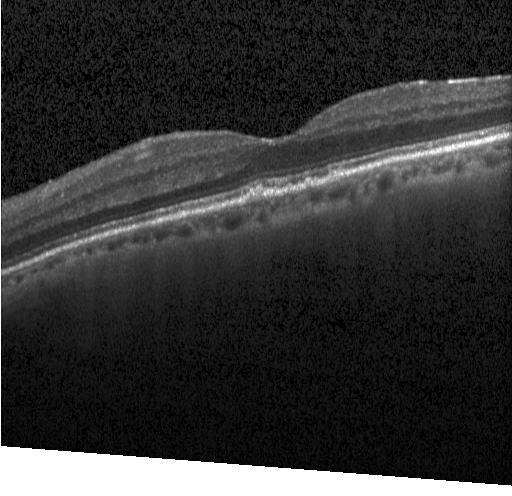 Optical coherence tomography B-scan. OCT finding: drusen.